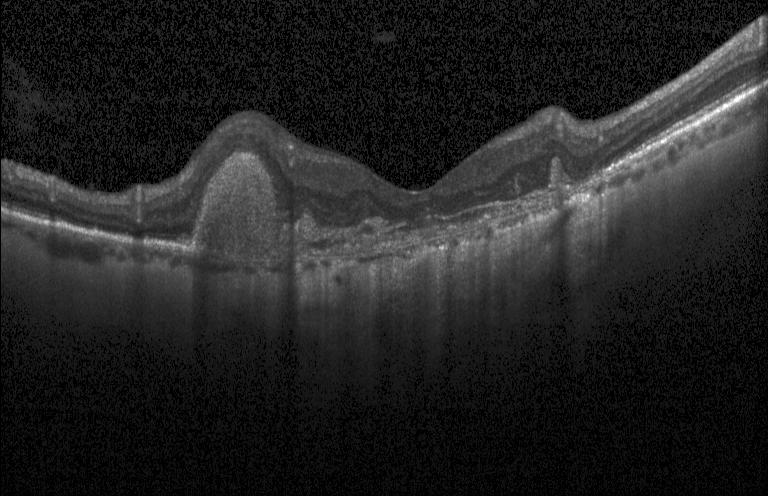
Diagnosis: a choroidal neovascular membrane.